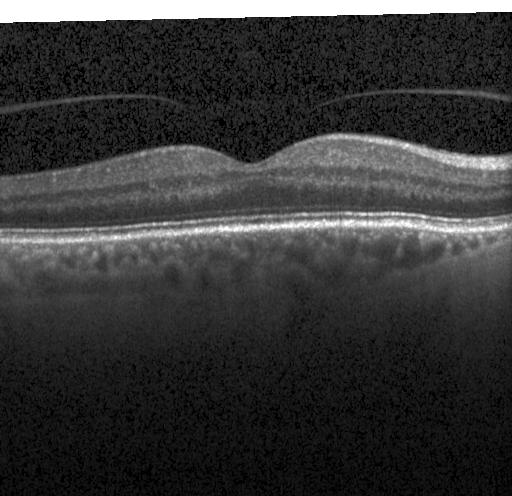
OCT B-scan — Finding: no choroidal neovascularization, no diabetic macular edema, and no drusen.